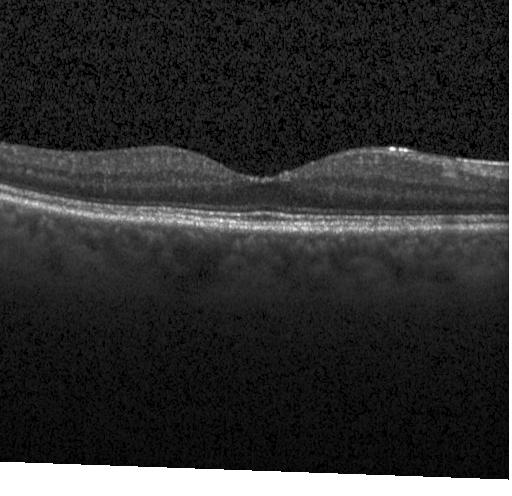 Dx: no CNV, DME, or drusen.